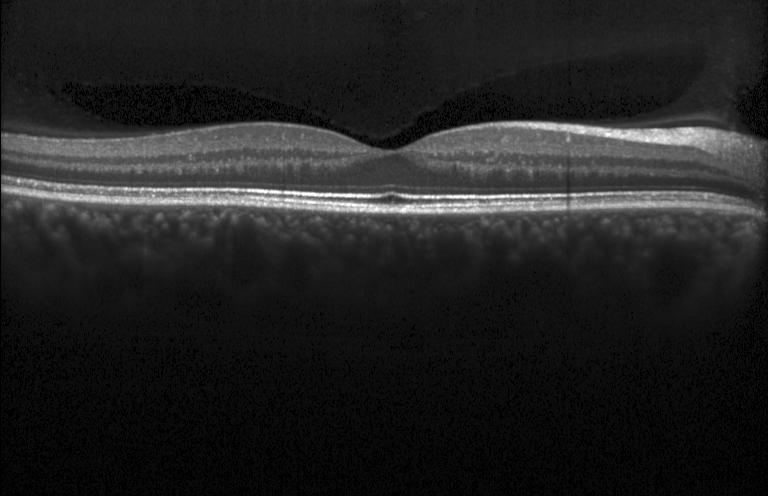
Optical coherence tomography scan
The scan shows no choroidal neovascularization, diabetic macular edema, or drusen.